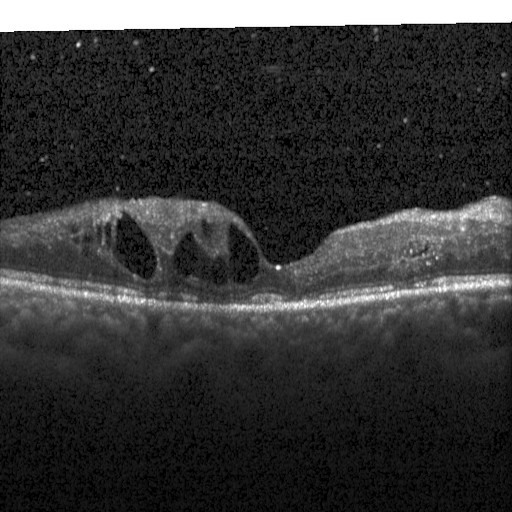 Heidelberg Spectralis. Optical coherence tomography scan.
Finding: diabetic macular edema (DME).